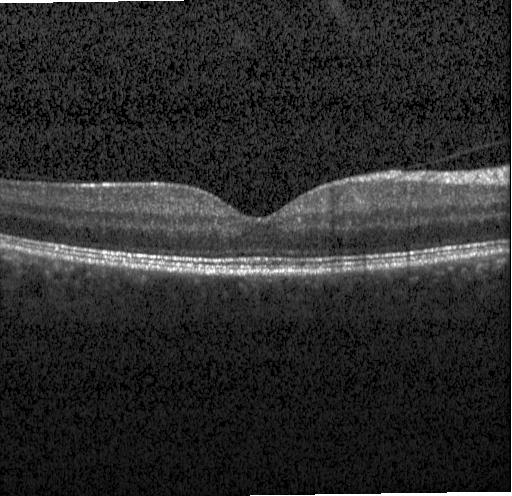 Retinal OCT B-scan.
Diagnosis: no CNV, DME, or drusen.